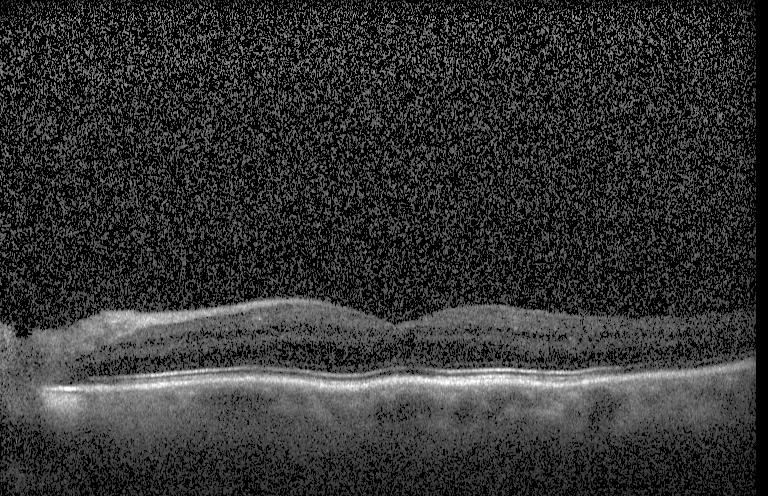 SD-OCT. OCT B-scan. Heidelberg Spectralis OCT system. Macular scan
Impression: no evidence of choroidal neovascularization, diabetic macular edema, or drusen.